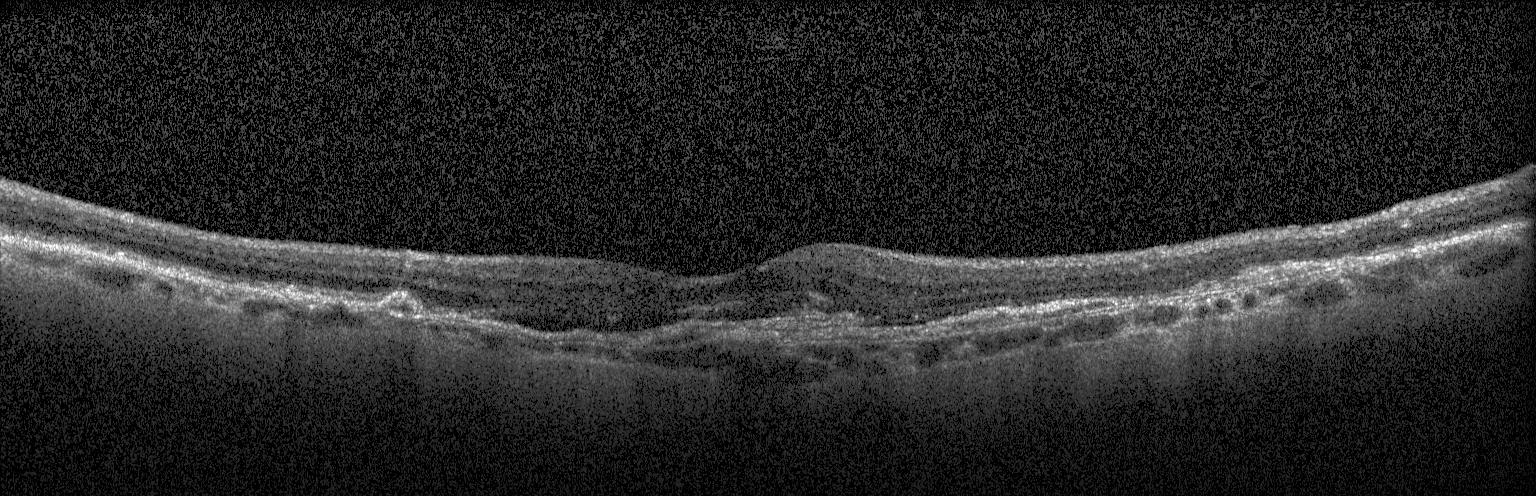
OCT finding: a choroidal neovascular membrane.